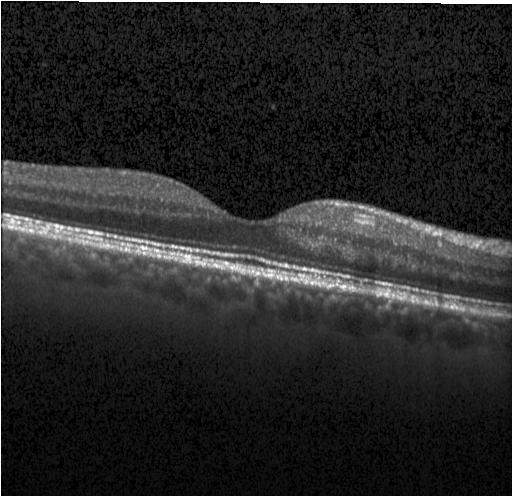

Impression: no evidence of CNV, DME, or drusen.